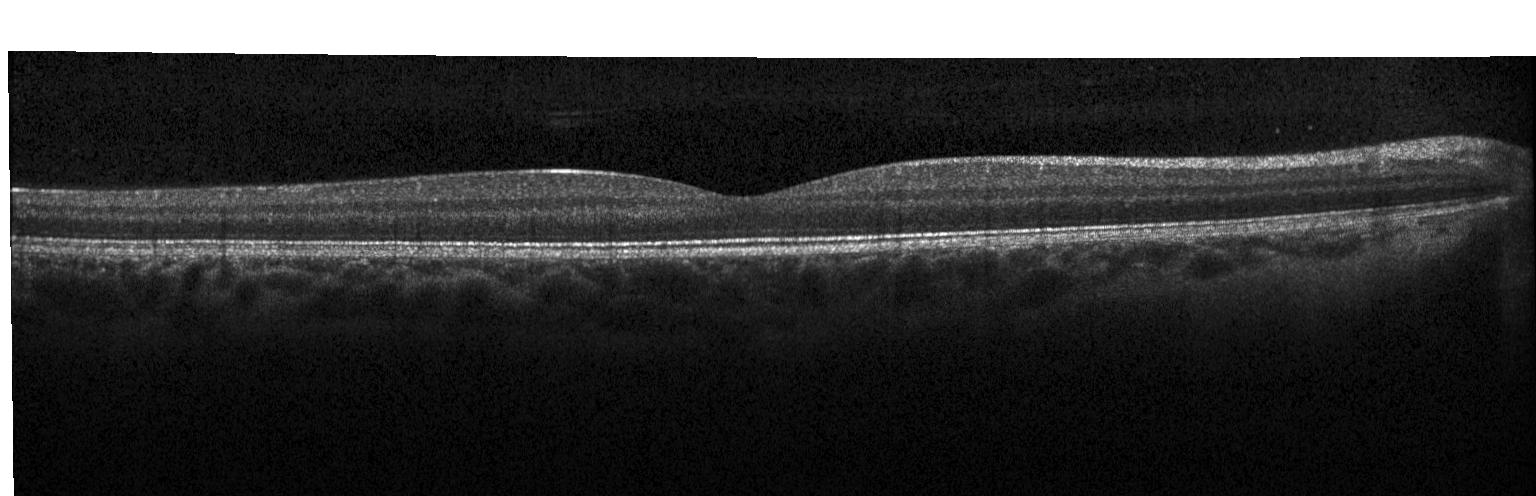 Retinal OCT cross-section showing no evidence of CNV, DME, or drusen.